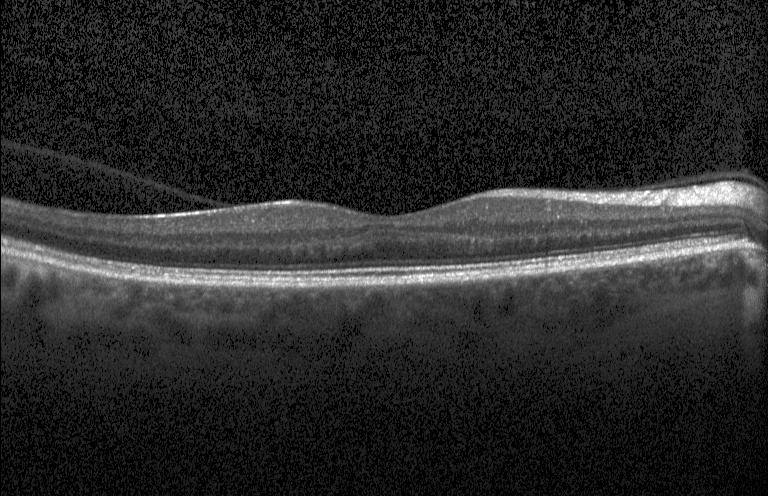
OCT scan showing no choroidal neovascularization, diabetic macular edema, or drusen.